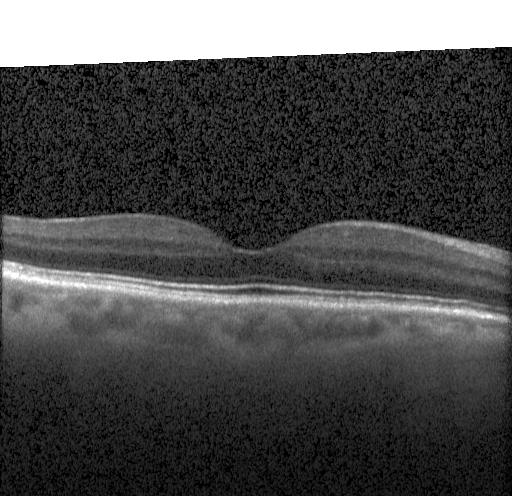 Spectral-domain optical coherence tomography · Heidelberg Spectralis OCT system · OCT line scan · fovea-centered. Impression: no choroidal neovascularization, diabetic macular edema, or drusen.